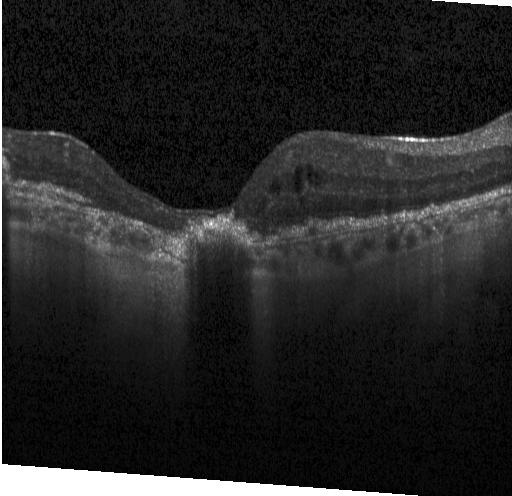

Centered on the fovea, OCT B-scan, spectral-domain optical coherence tomography — Finding: choroidal neovascularization (CNV).